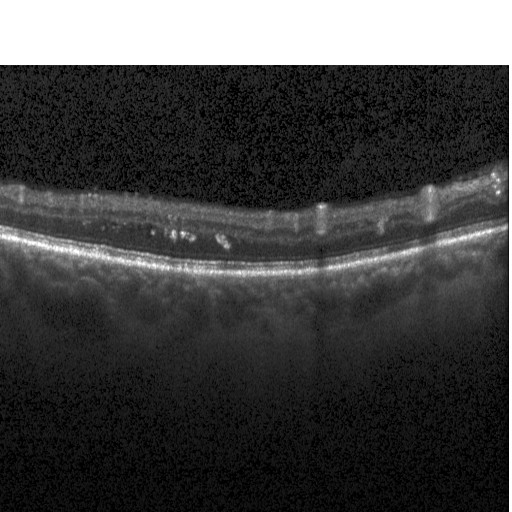
Impression: diabetic macular edema.